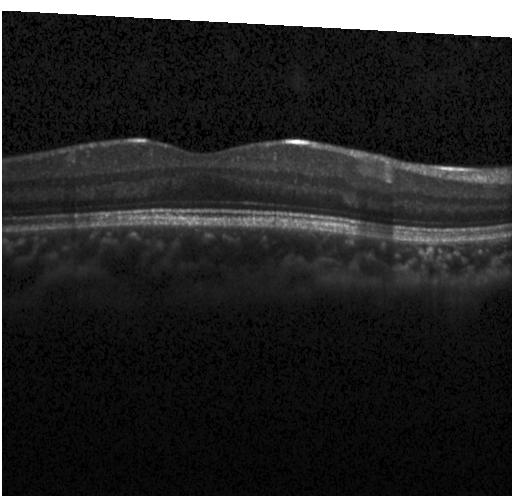 OCT B-scan, spectral-domain OCT, acquired on a Heidelberg Spectralis, centered on the fovea.
Finding: no evidence of choroidal neovascularization, diabetic macular edema, or drusen.